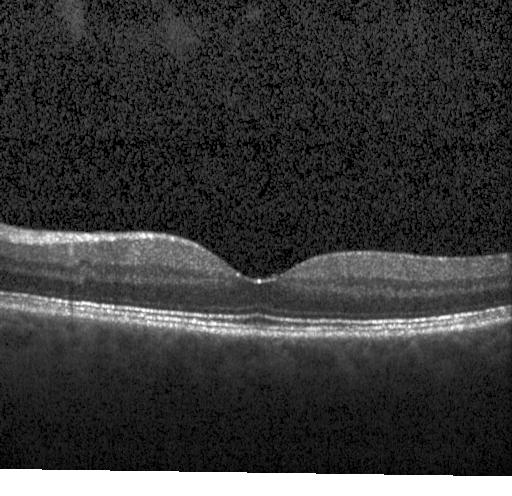
Spectral-domain OCT · OCT B-scan · centered on the fovea — Impression: neither CNV, DME, nor drusen.